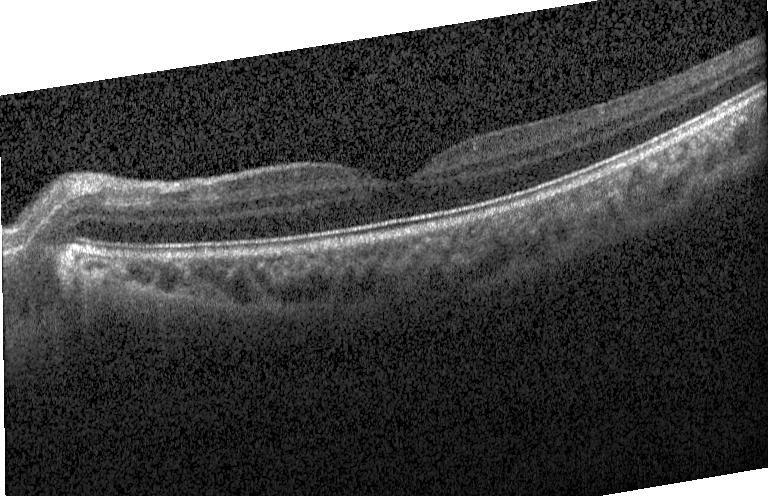

Macular OCT demonstrating no CNV, no DME, and no drusen.